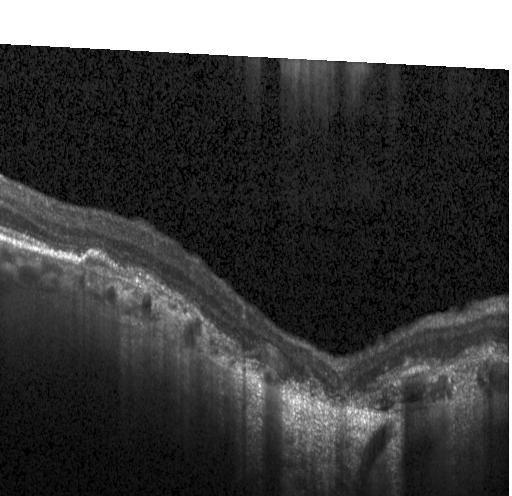

Diagnosis: choroidal neovascularization (CNV).